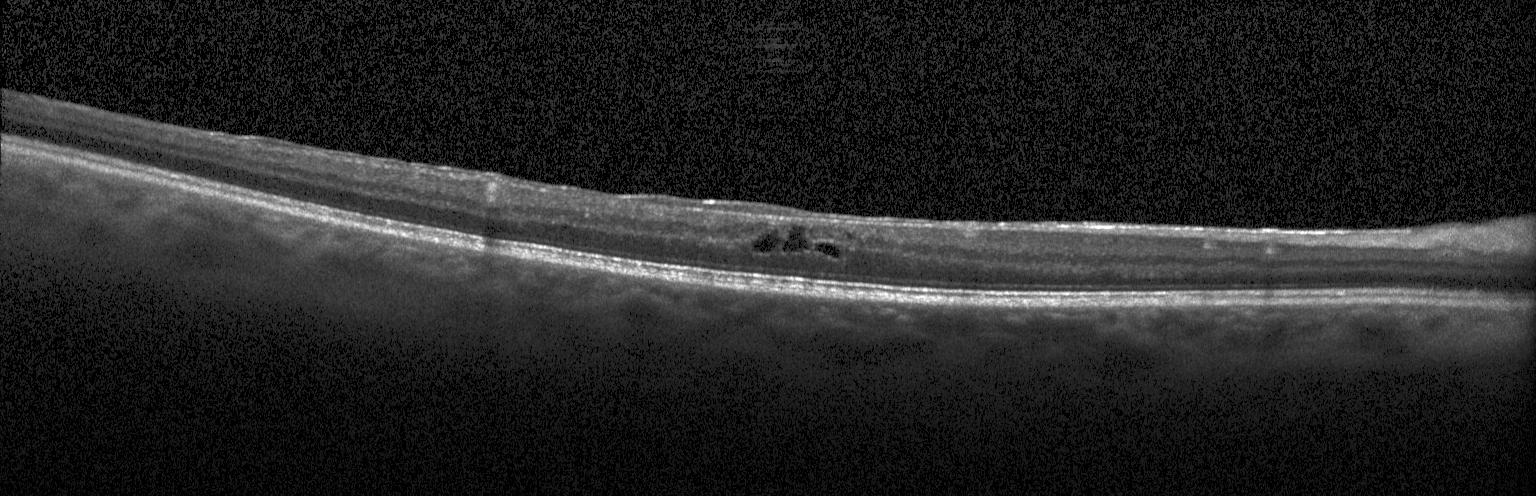 Diagnosis: DME.